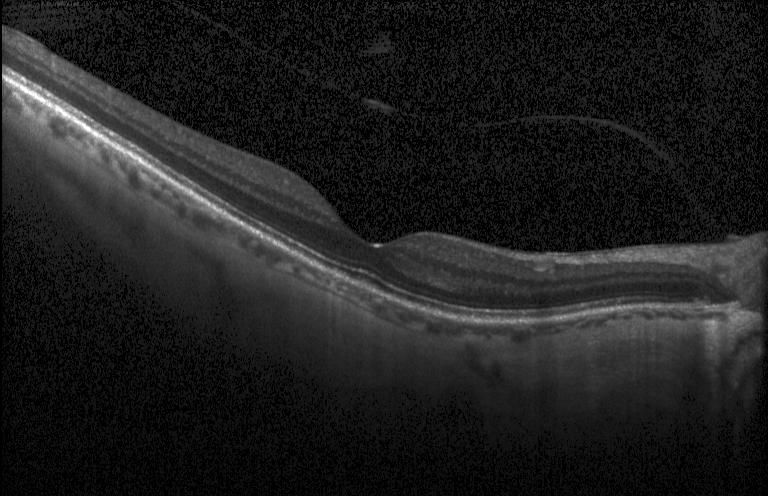
Retinal OCT cross-section. Dx: no choroidal neovascularization, diabetic macular edema, or drusen.